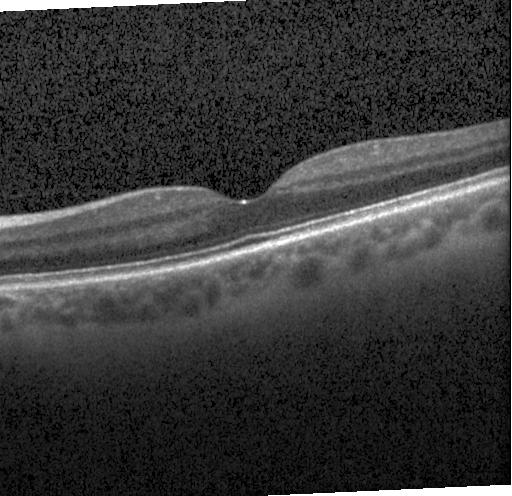 Retinal OCT cross-section
Assessment: no evidence of choroidal neovascularization, diabetic macular edema, or drusen.